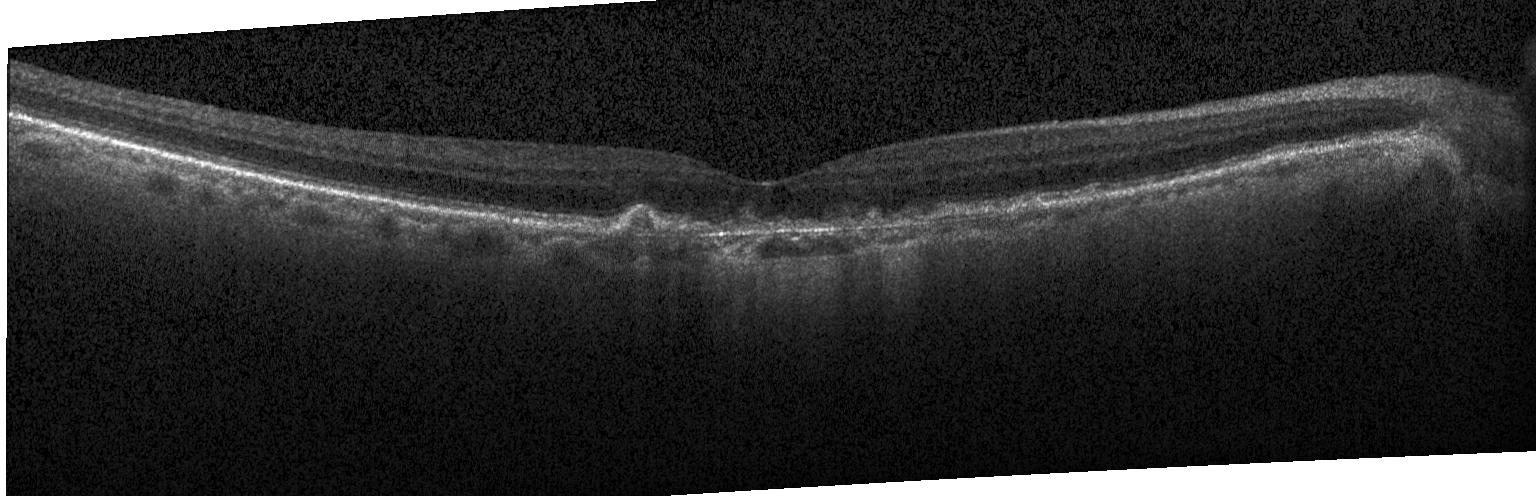 OCT B-scan; Heidelberg Spectralis; horizontal scan through the fovea; spectral-domain optical coherence tomography. A choroidal neovascular membrane.